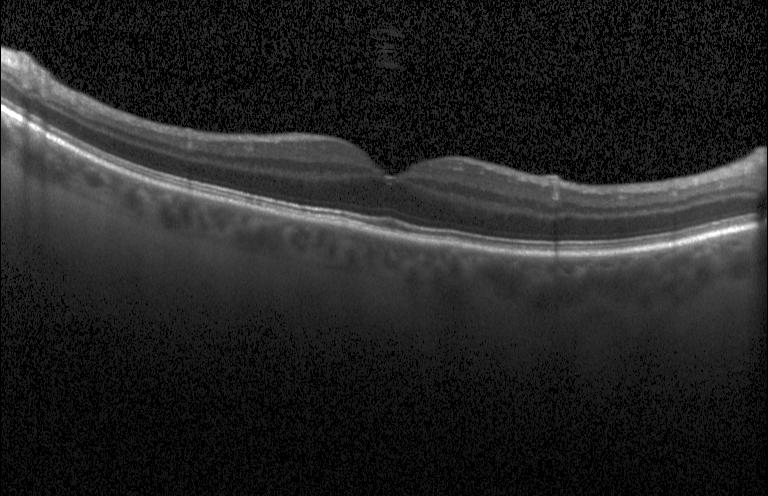
Retinal OCT B-scan — OCT finding: no choroidal neovascularization, diabetic macular edema, or drusen.